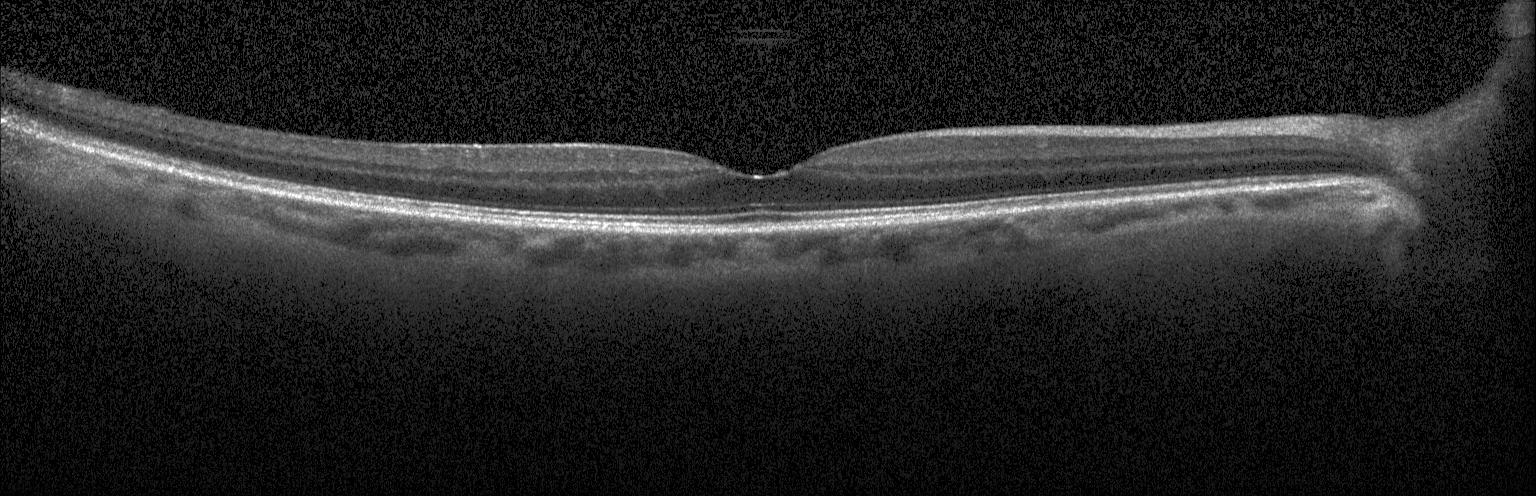
Through the macula. Retinal OCT cross-section. Diagnosis: no CNV, DME, or drusen.